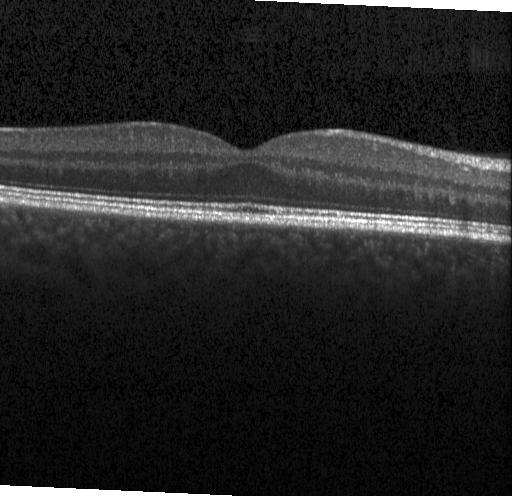

SD-OCT. Optical coherence tomography scan. Heidelberg Spectralis OCT system. Fovea-centered.
The scan shows no choroidal neovascularization, diabetic macular edema, or drusen.